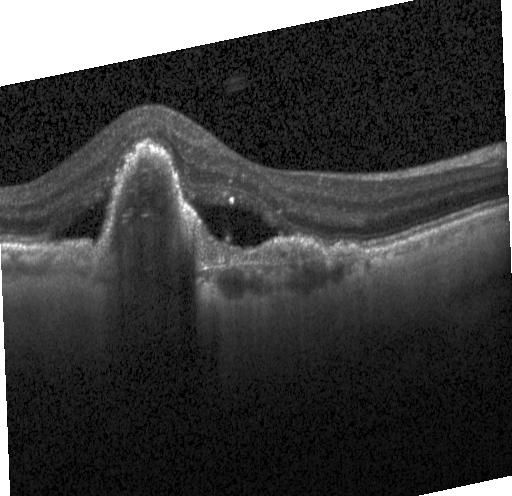
Heidelberg Spectralis OCT system, spectral-domain OCT, retinal OCT B-scan.
Diagnosis: a choroidal neovascular membrane.